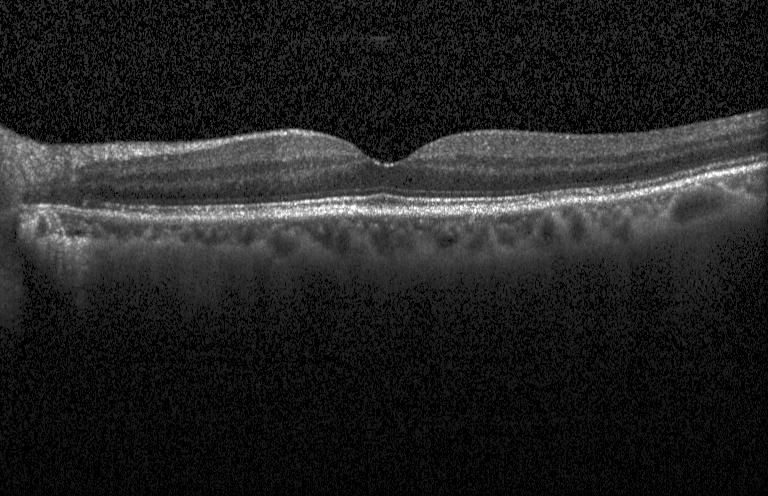

Through the macula, retinal OCT B-scan.
Impression: no choroidal neovascularization, no diabetic macular edema, and no drusen.